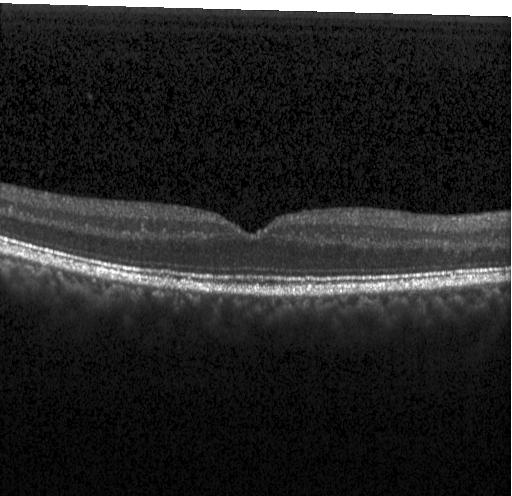 Macular OCT: no evidence of choroidal neovascularization, diabetic macular edema, or drusen.